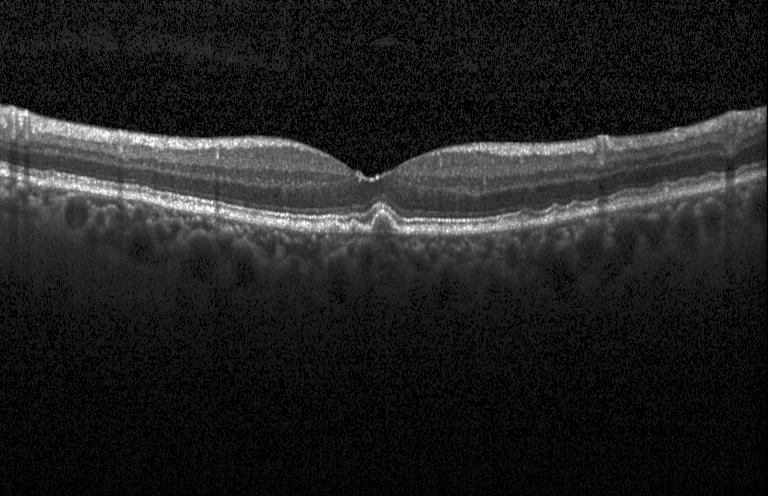
Macular scan. Instrument: Heidelberg Spectralis. Optical coherence tomography B-scan.
Assessment: multiple drusen.